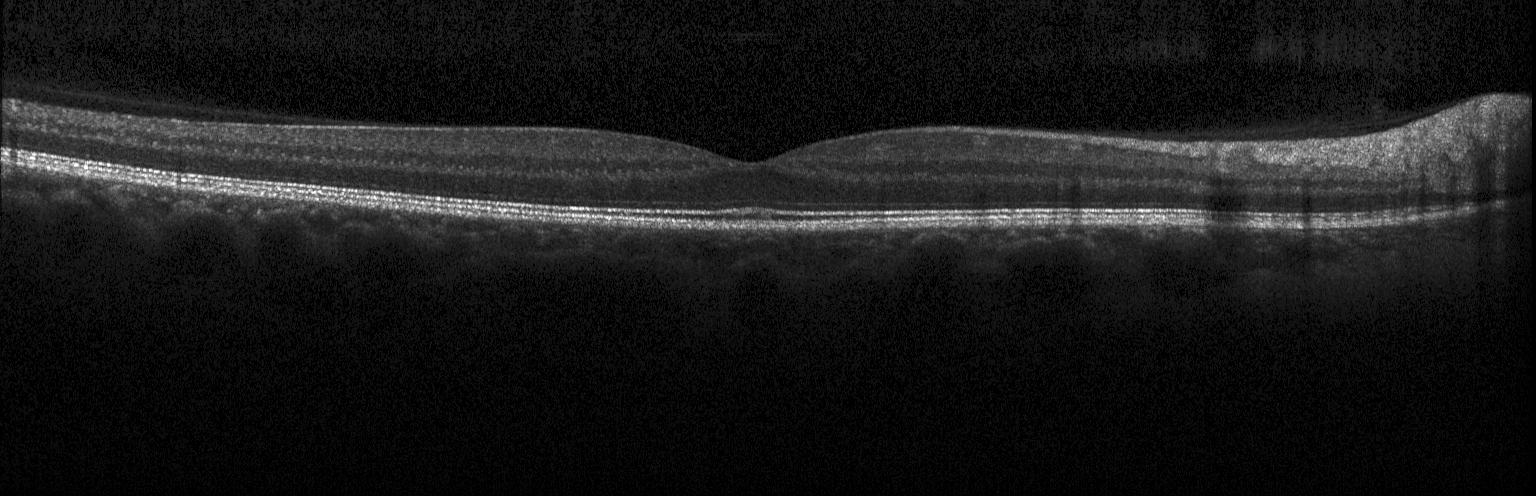
Spectral-domain OCT. Retinal OCT B-scan — Dx: no choroidal neovascularization, no diabetic macular edema, and no drusen.